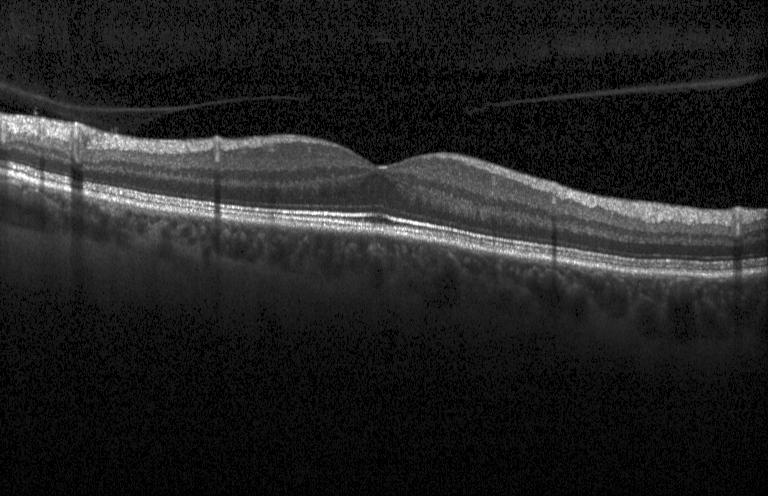

OCT finding: no choroidal neovascularization, diabetic macular edema, or drusen.